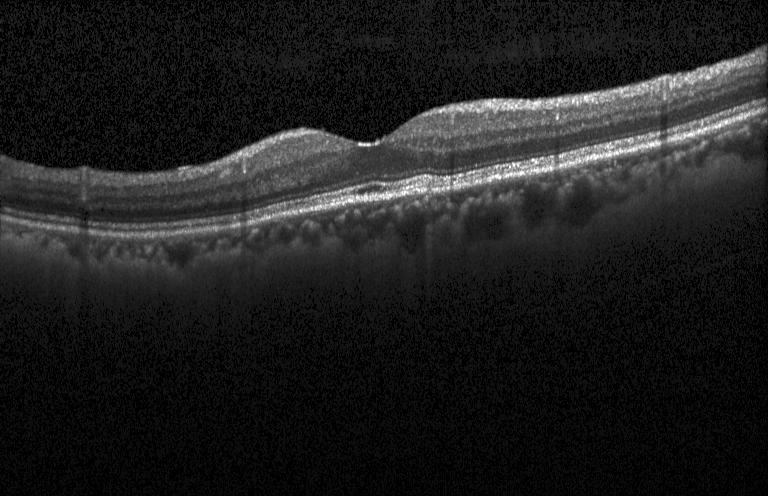

OCT finding: no evidence of CNV, DME, or drusen.